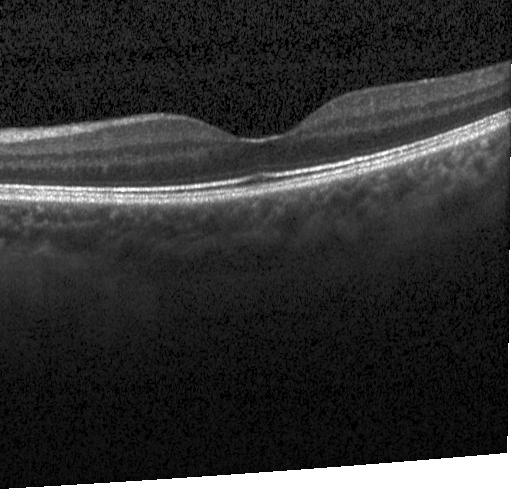

Optical coherence tomography scan; Heidelberg Spectralis; spectral-domain OCT; macular scan — Diagnosis: no evidence of CNV, DME, or drusen.